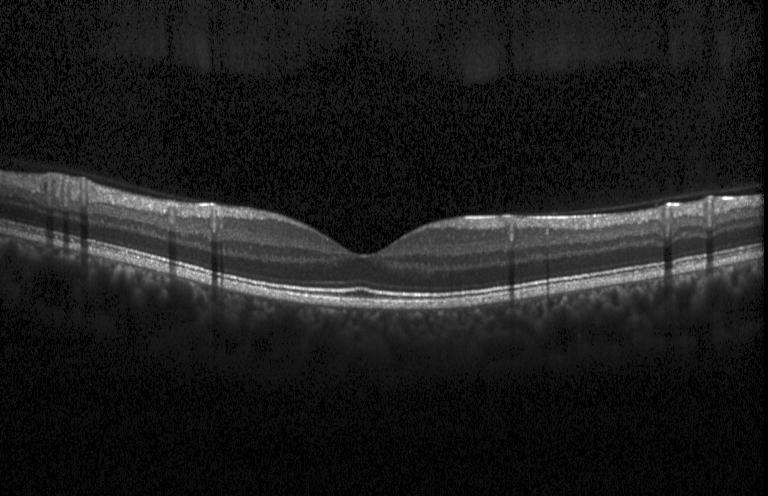 Macular OCT: neither CNV, DME, nor drusen.